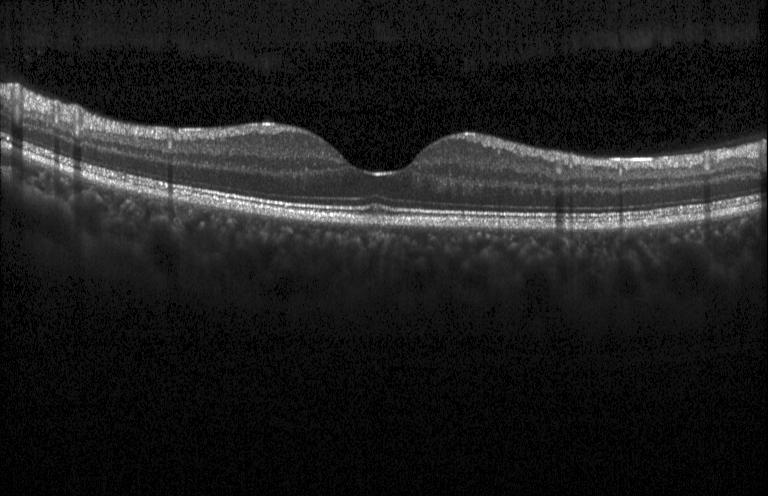
The scan shows no CNV, no DME, and no drusen.